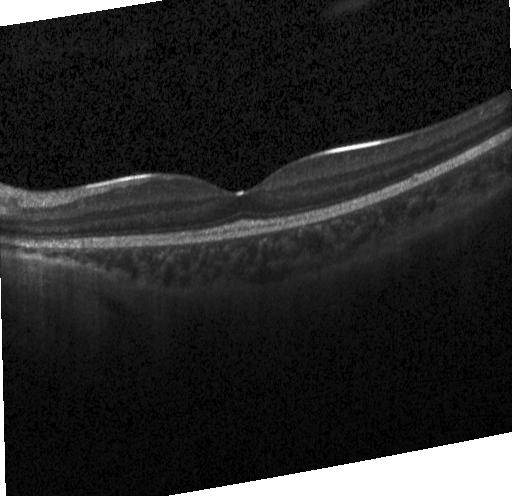 Macular scan, instrument: Heidelberg Spectralis, spectral-domain OCT, optical coherence tomography B-scan.
Finding: no evidence of CNV, DME, or drusen.